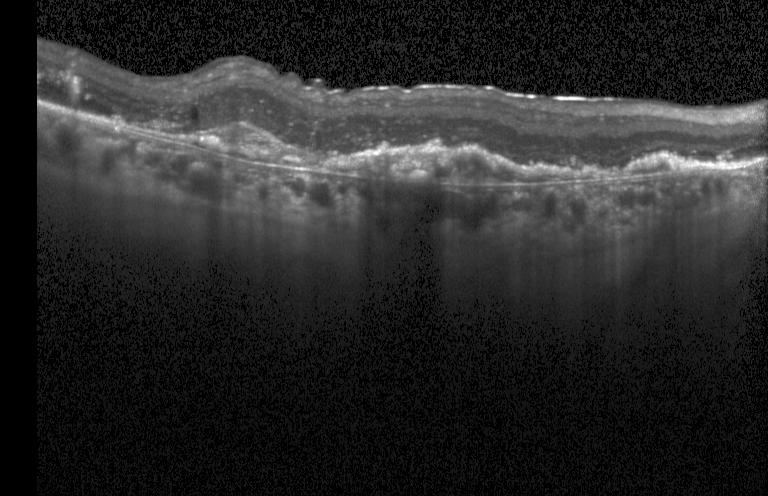 The scan shows choroidal neovascularization (CNV).